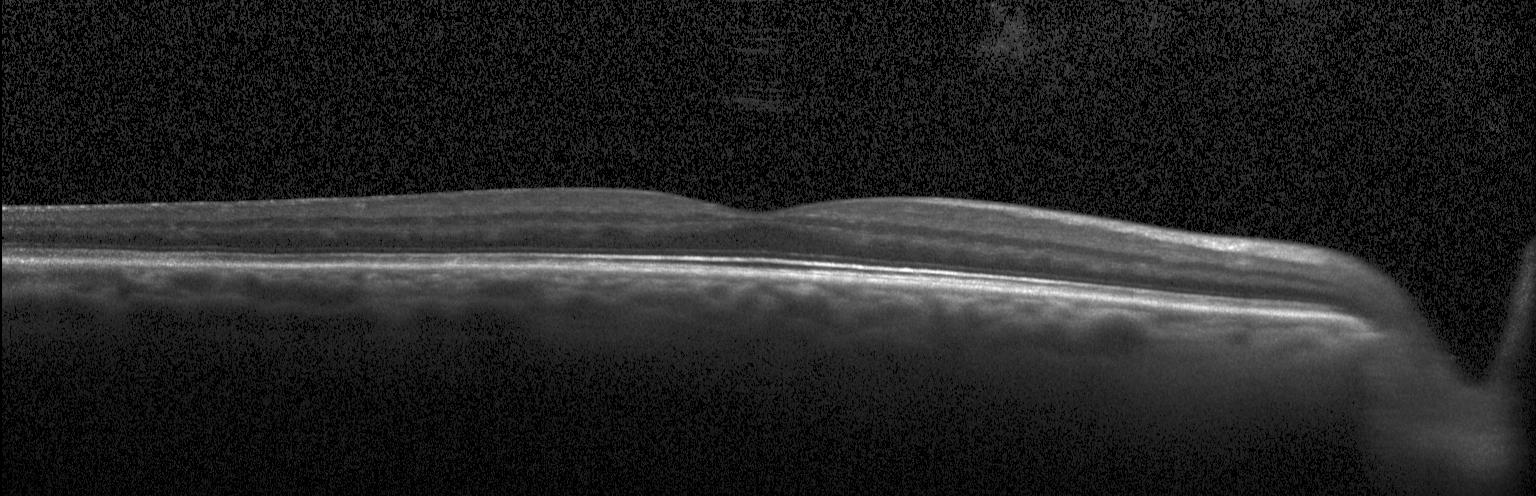 Centered on the fovea. Optical coherence tomography B-scan. Spectral-domain optical coherence tomography.
Finding: no choroidal neovascularization, diabetic macular edema, or drusen.